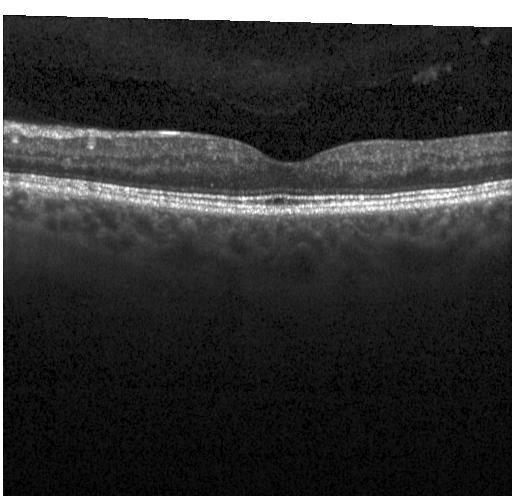

Retinal OCT B-scan.
This B-scan demonstrates no evidence of choroidal neovascularization, diabetic macular edema, or drusen.